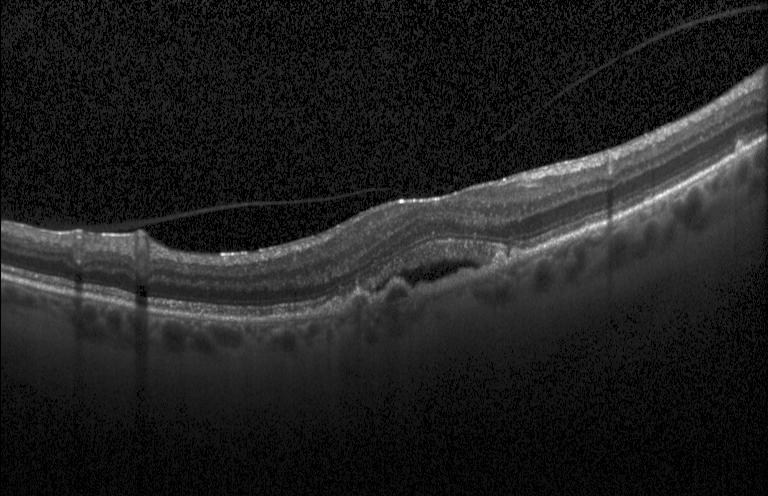
Optical coherence tomography B-scan. Acquired on a Heidelberg Spectralis. Centered on the fovea. SD-OCT. A choroidal neovascular membrane.